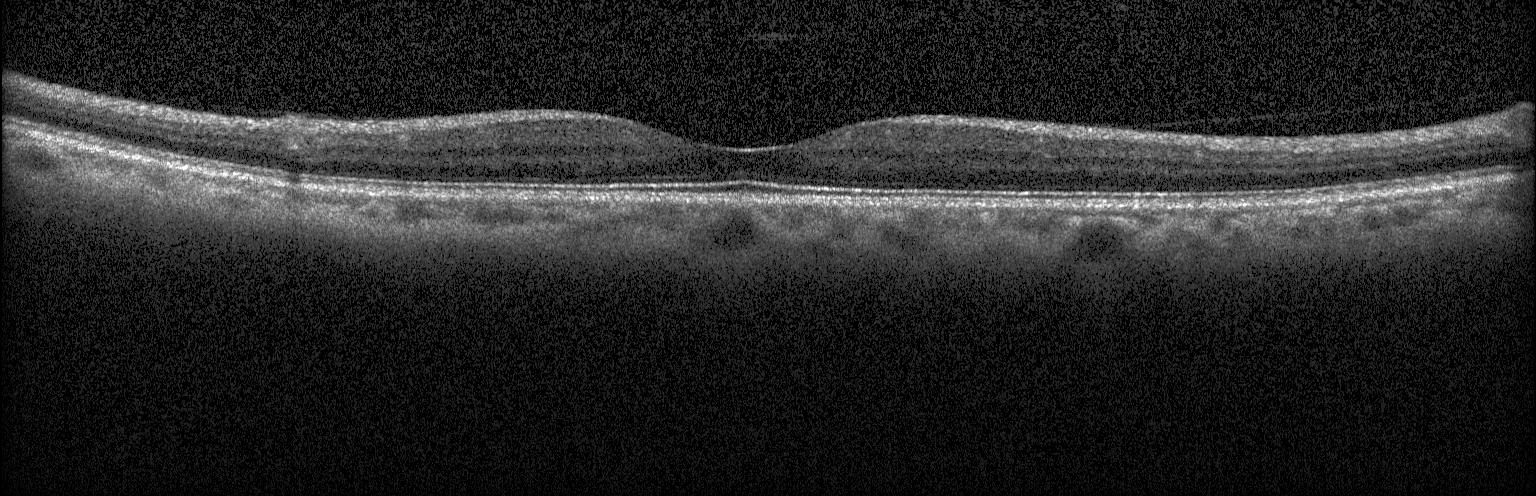

Retinal OCT cross-section
Macular OCT: no CNV, DME, or drusen.